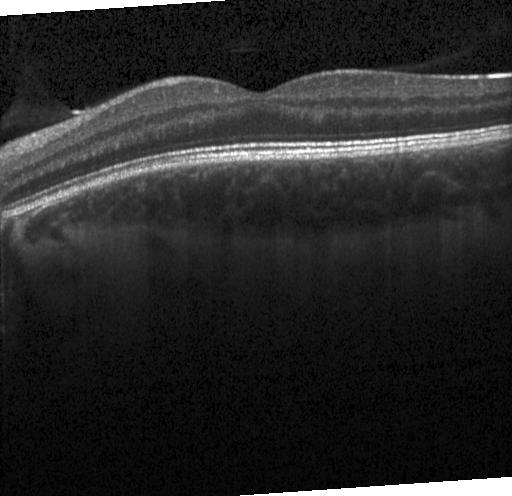
OCT line scan — Diagnosis: no choroidal neovascularization, diabetic macular edema, or drusen.